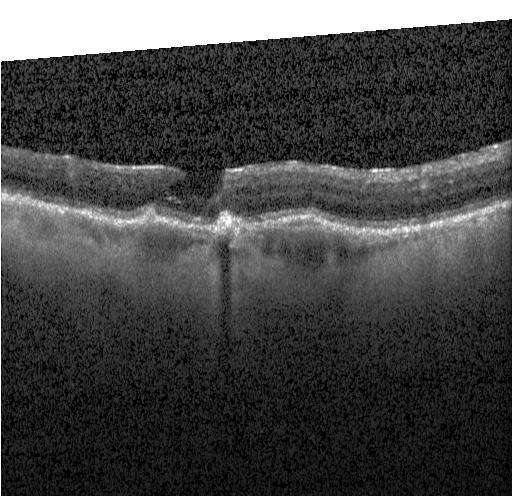

Retinal OCT B-scan
Dx: choroidal neovascularization.